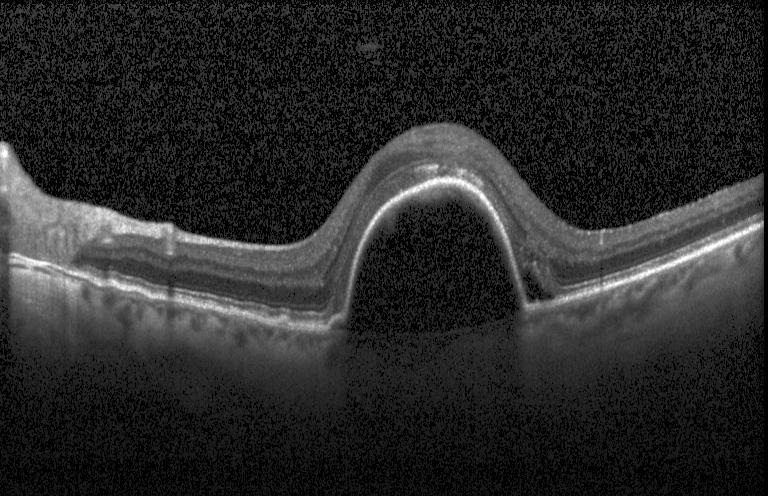
Through the macula. Optical coherence tomography scan. Impression: a choroidal neovascular membrane.